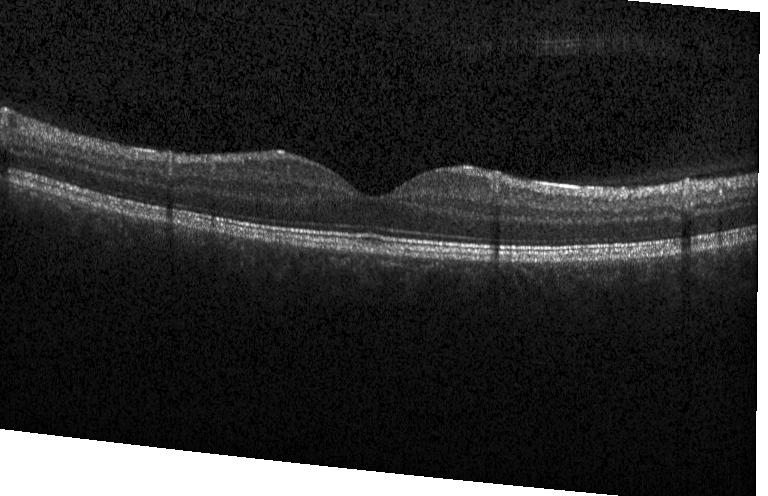 Impression: no choroidal neovascularization, no diabetic macular edema, and no drusen.